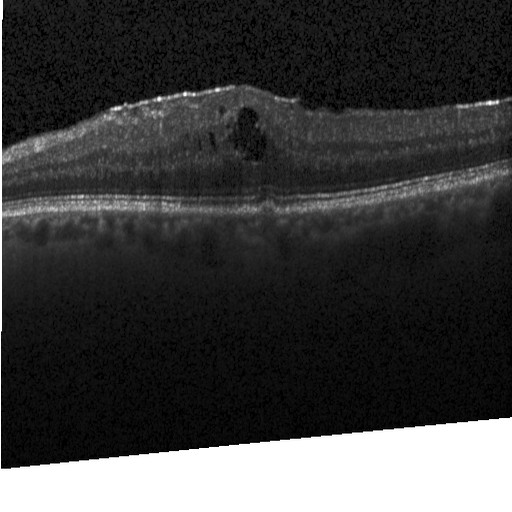
Diagnosis: DME.